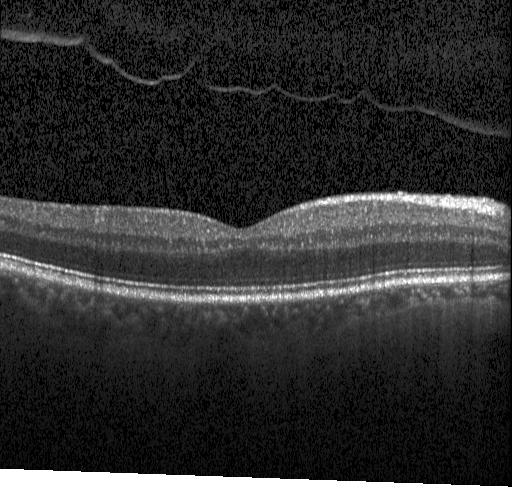

Assessment: no choroidal neovascularization, no diabetic macular edema, and no drusen.